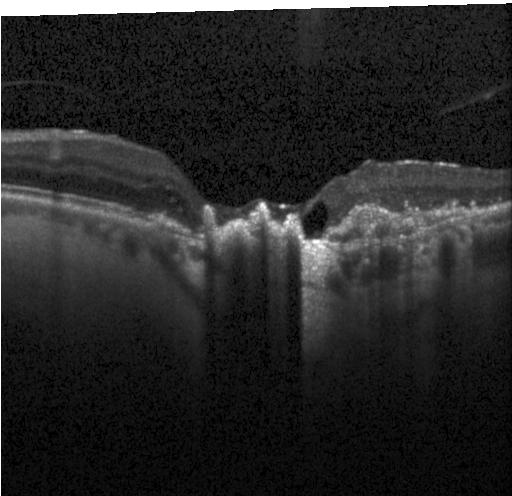

OCT scan showing a choroidal neovascular membrane.